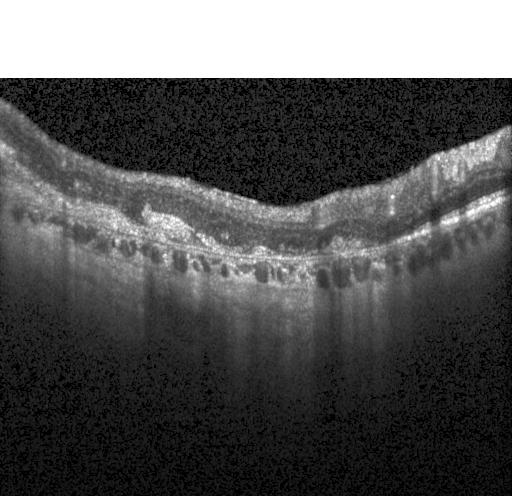

Centered on the fovea · OCT B-scan · SD-OCT · Heidelberg Spectralis OCT system — Finding: choroidal neovascularization (CNV).